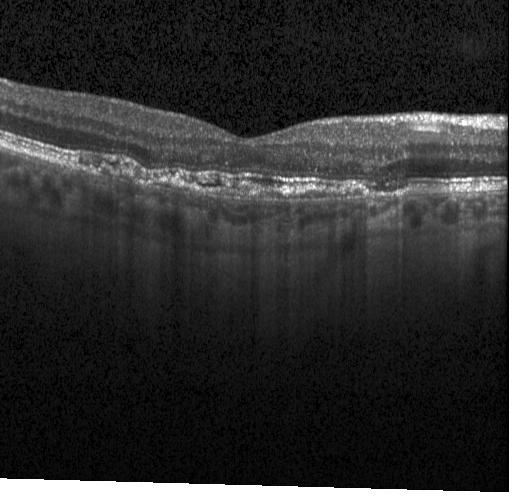 OCT scan showing a choroidal neovascular membrane.